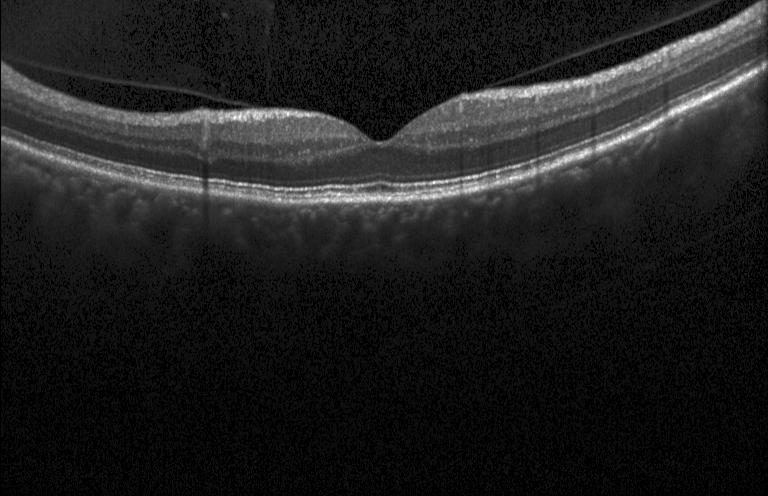

SD-OCT. Centered on the fovea. Acquired on a Heidelberg Spectralis. Retinal OCT B-scan. Diagnosis: no CNV, no DME, and no drusen.